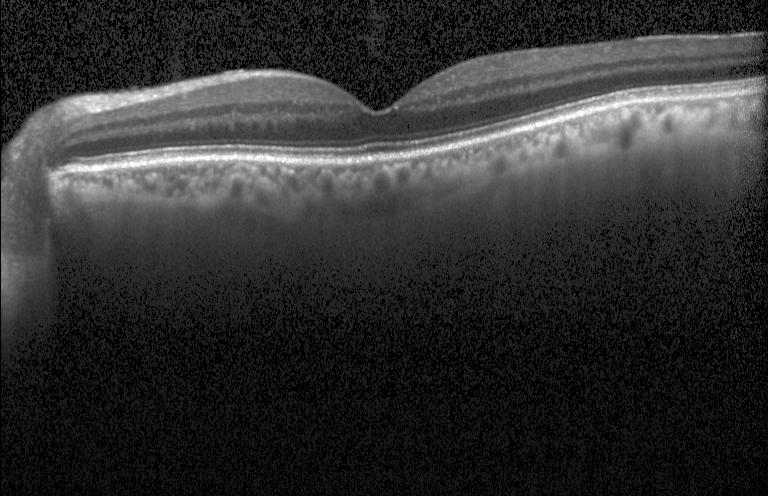 Spectral-domain optical coherence tomography, macular scan, retinal OCT cross-section.
The scan shows neither choroidal neovascularization, diabetic macular edema, nor drusen.